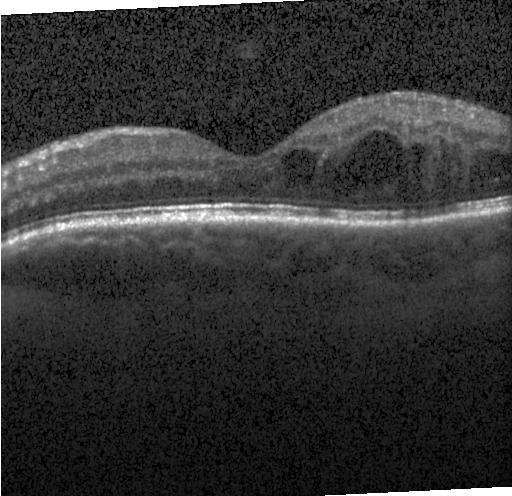
Retinal OCT cross-section showing diabetic macular edema.